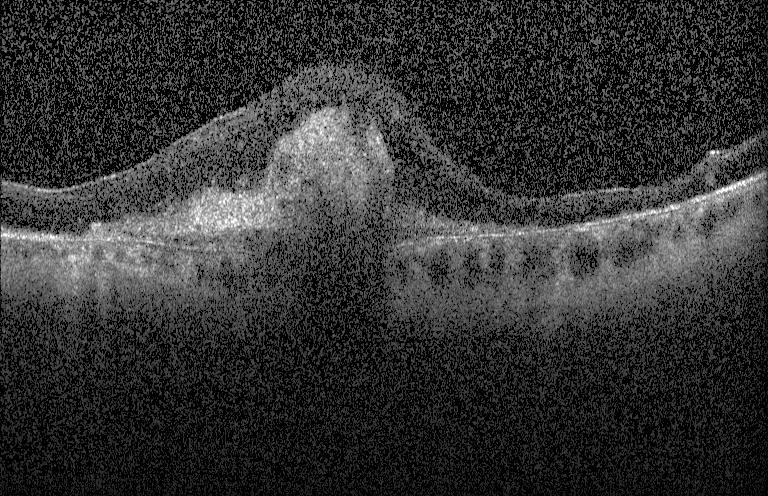
Horizontal scan through the fovea. Instrument: Heidelberg Spectralis. Spectral-domain OCT. Retinal OCT B-scan. Diagnosis: CNV.